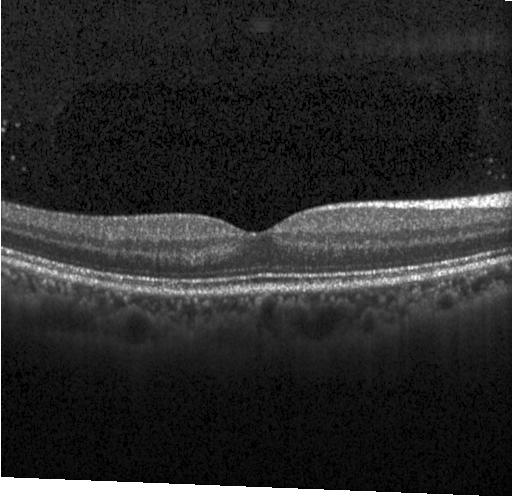 Spectral-domain OCT; OCT B-scan.
The scan shows no choroidal neovascularization, no diabetic macular edema, and no drusen.